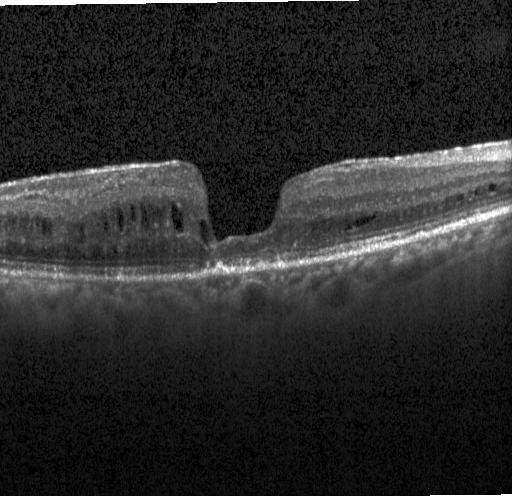 Spectral-domain OCT. Macular scan. Acquired on a Heidelberg Spectralis. Retinal OCT cross-section.
Impression: DME.